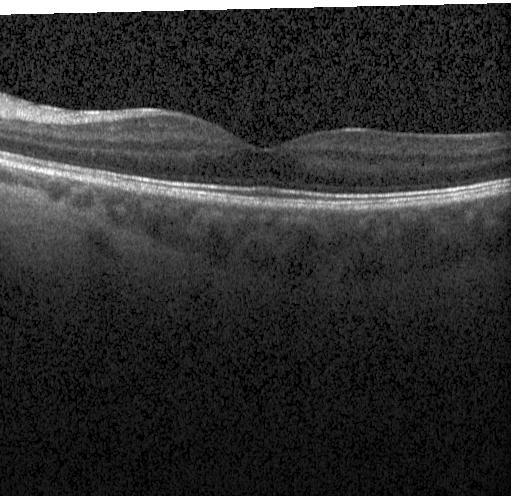

Finding: no CNV, no DME, and no drusen.